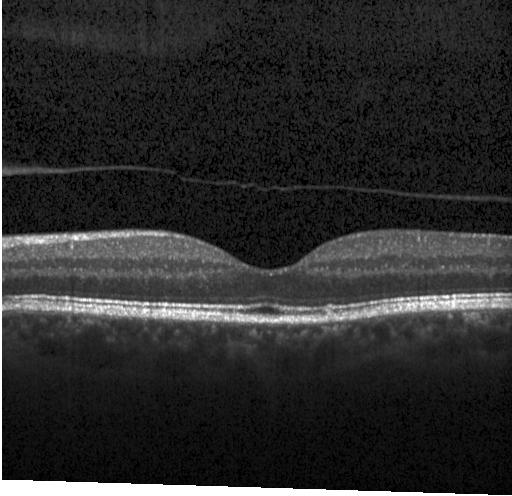

Diagnosis: no evidence of choroidal neovascularization, diabetic macular edema, or drusen.